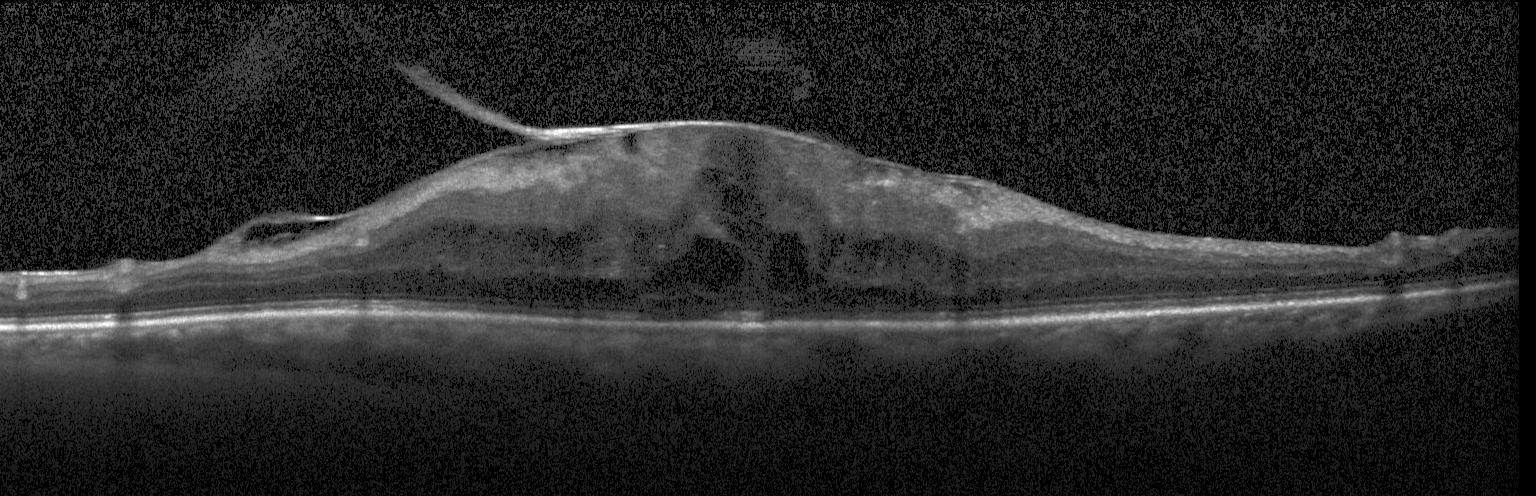
Spectral-domain OCT B-scan: DME.